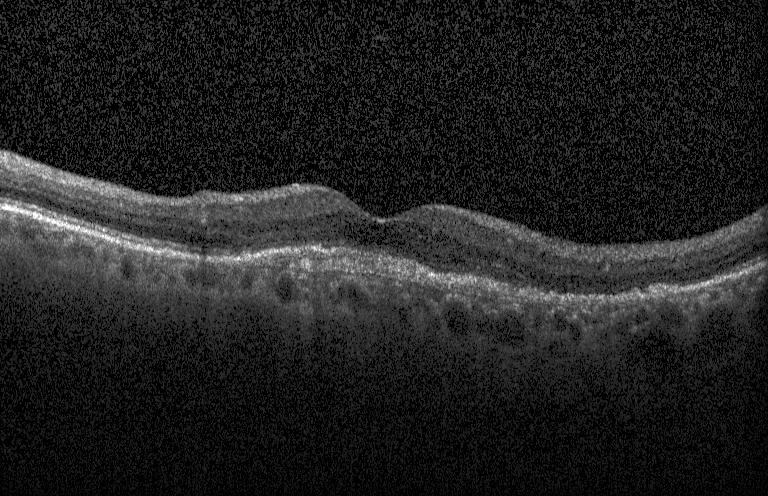 OCT B-scan.
Choroidal neovascularization (CNV).